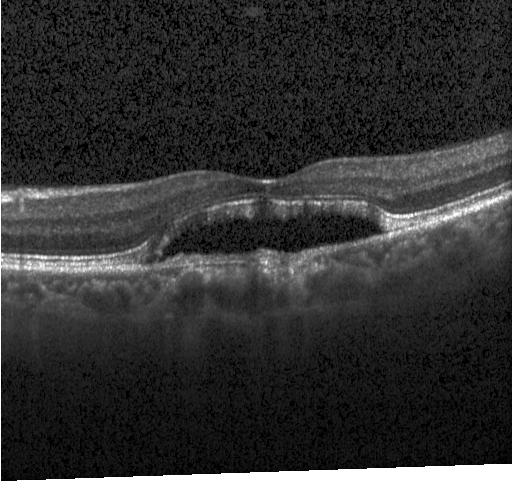
Finding: a choroidal neovascular membrane.